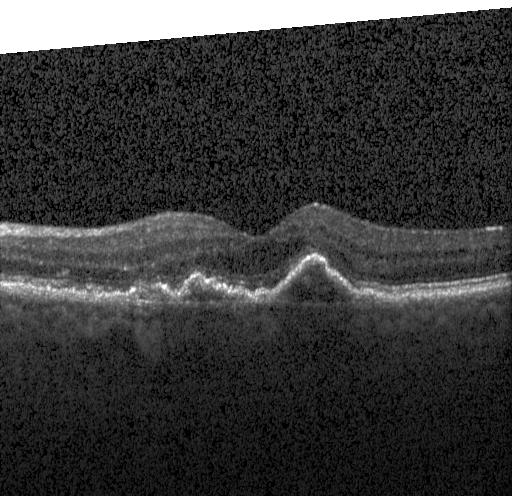

Macular scan; acquired on a Heidelberg Spectralis; OCT B-scan
Impression: choroidal neovascularization.